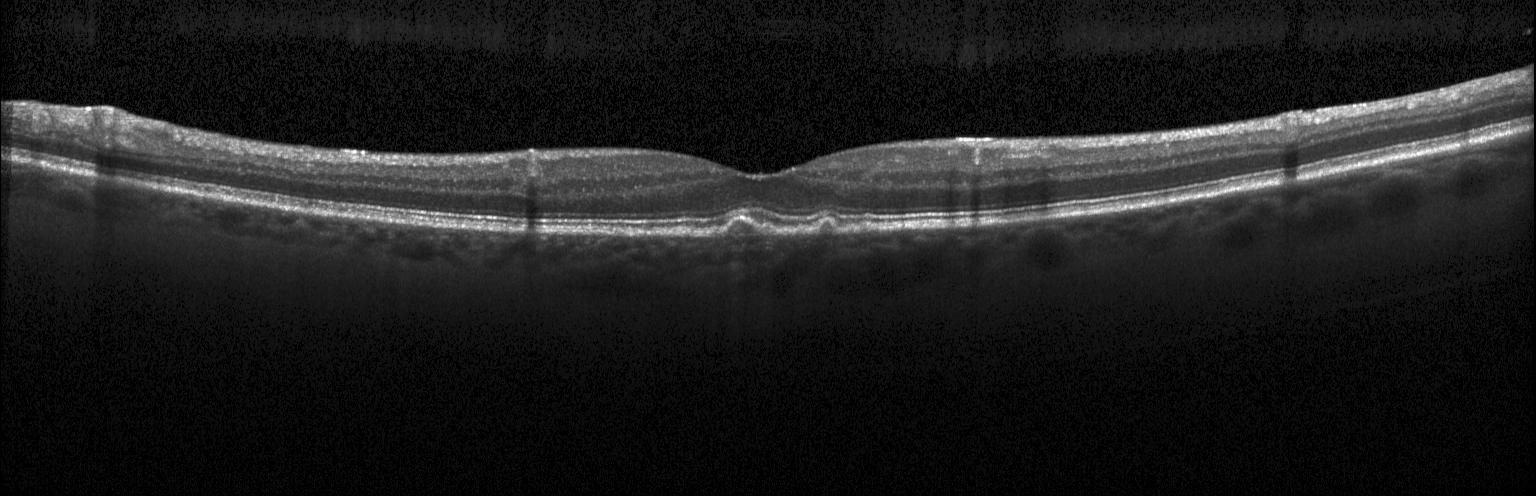
Spectral-domain optical coherence tomography. OCT line scan. Heidelberg Spectralis OCT system. Diagnosis: sub-RPE drusenoid deposits.